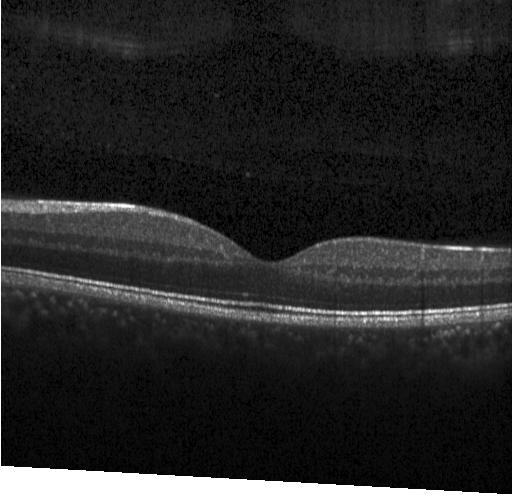
OCT scan showing neither choroidal neovascularization, diabetic macular edema, nor drusen.